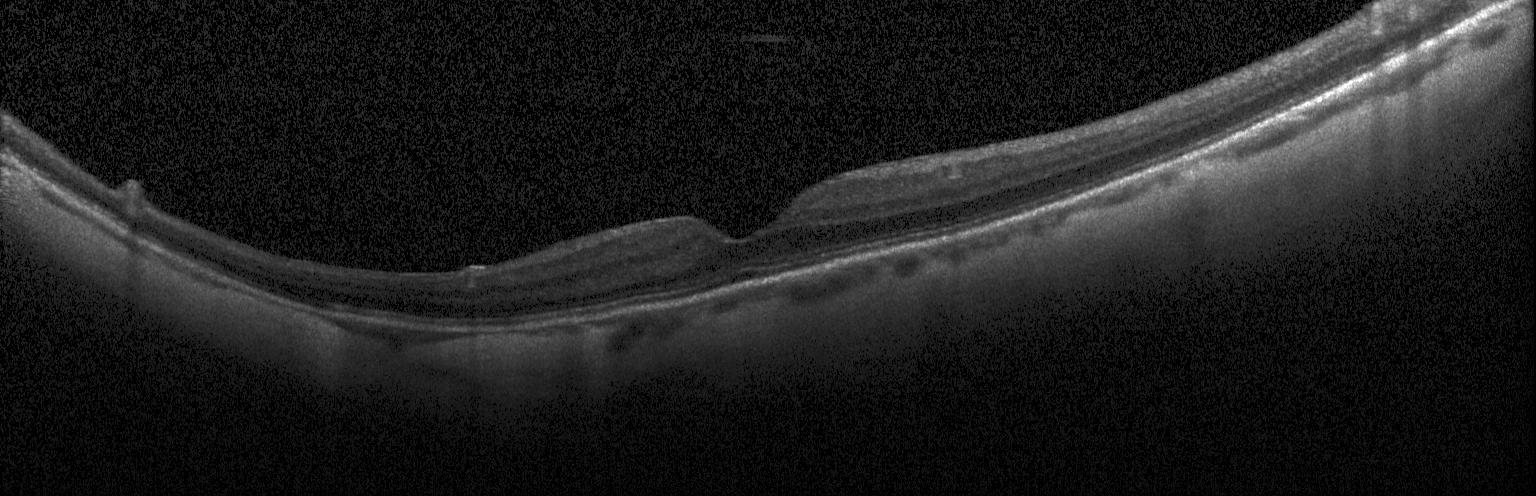

Spectral-domain OCT B-scan: no choroidal neovascularization, no diabetic macular edema, and no drusen.